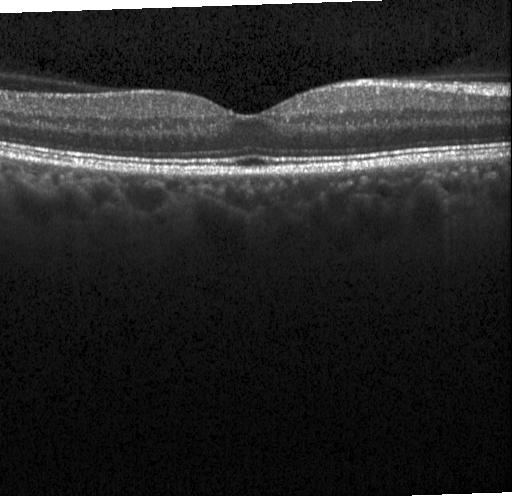 Diagnosis: no CNV, DME, or drusen.